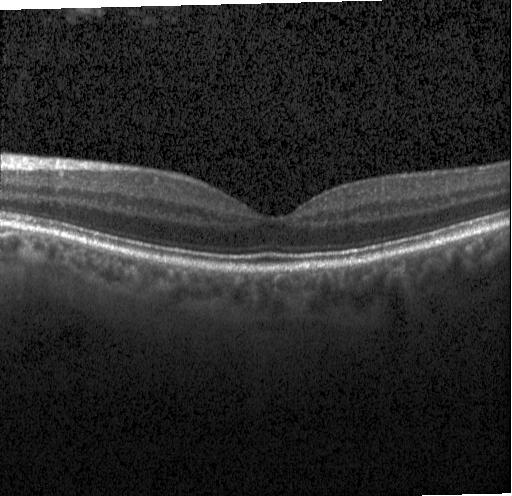

Diagnosis: no CNV, no DME, and no drusen.